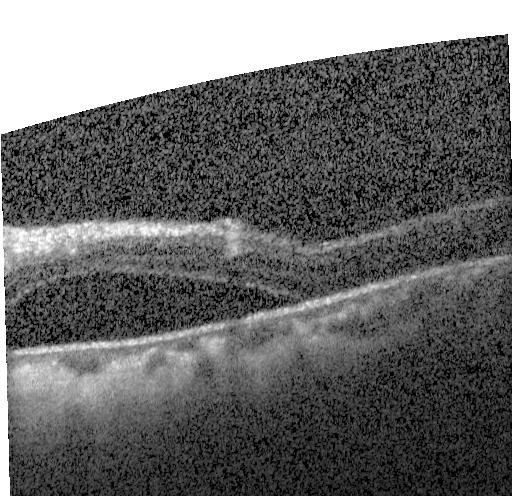

SD-OCT; instrument: Heidelberg Spectralis; OCT B-scan. Finding: choroidal neovascularization.